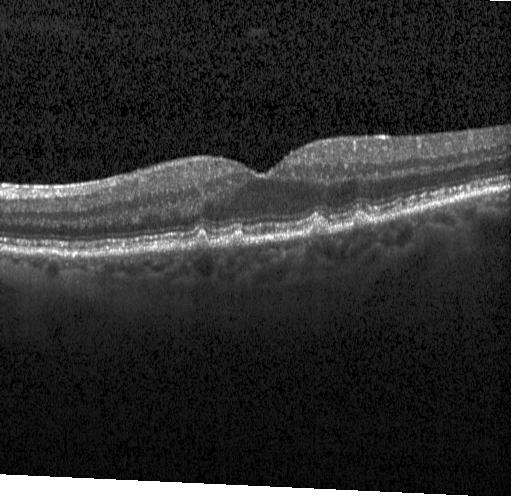

Retinal OCT cross-section. Impression: multiple drusen.